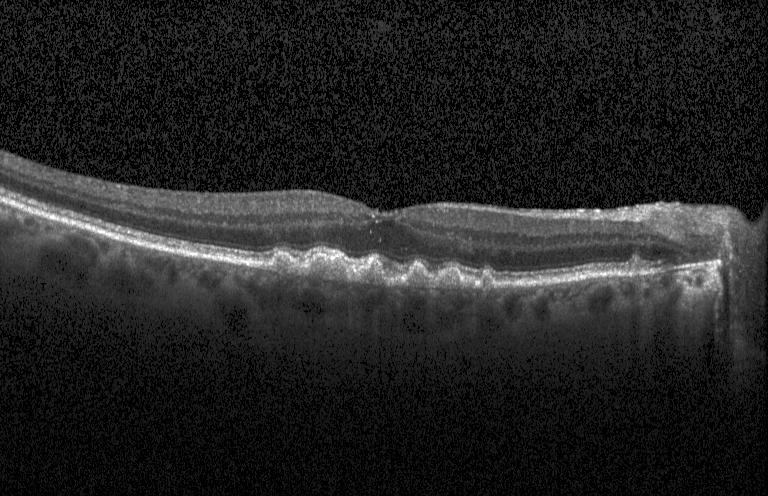

Macular scan. Retinal OCT B-scan — Multiple drusen.